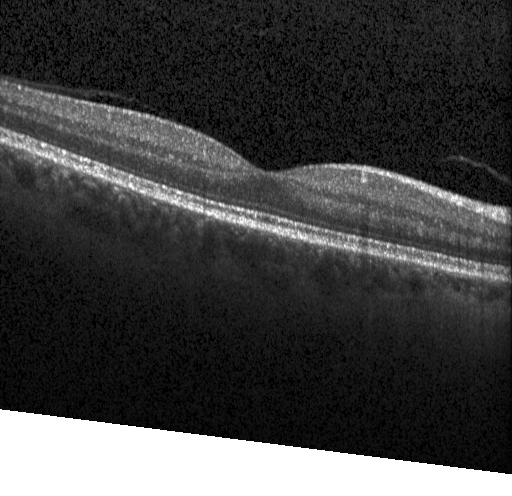

This B-scan demonstrates no choroidal neovascularization, no diabetic macular edema, and no drusen.